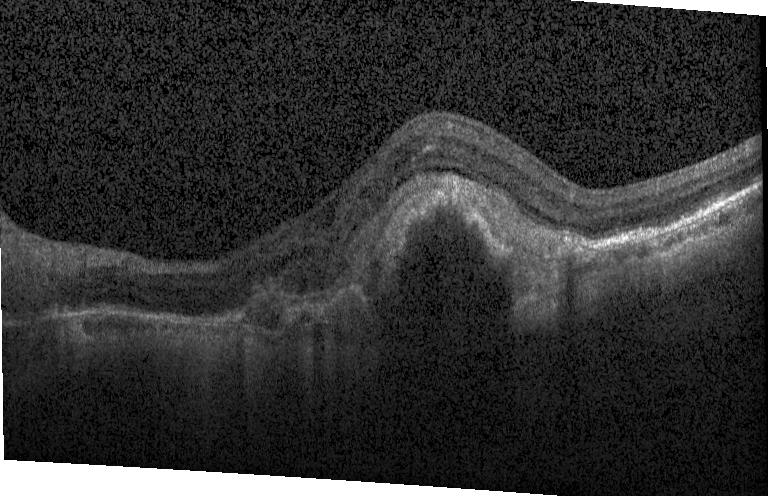
Retinal OCT cross-section showing choroidal neovascularization.